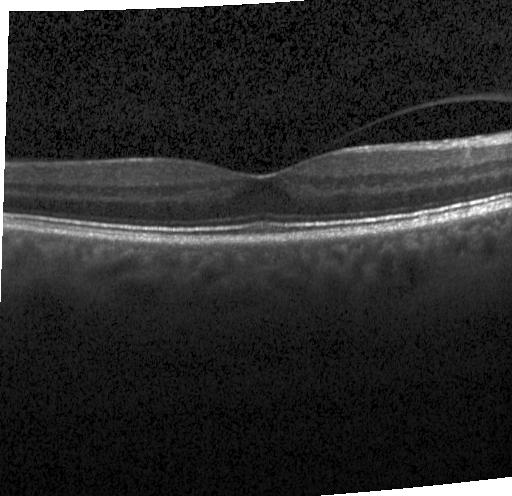 Heidelberg Spectralis OCT system; OCT B-scan.
Finding: no choroidal neovascularization, diabetic macular edema, or drusen.